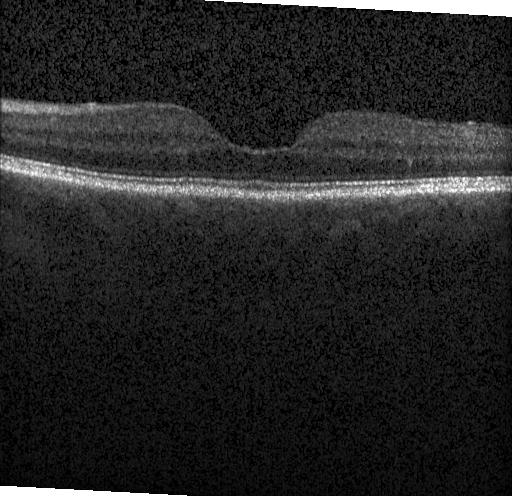

OCT B-scan. This B-scan demonstrates no evidence of choroidal neovascularization, diabetic macular edema, or drusen.